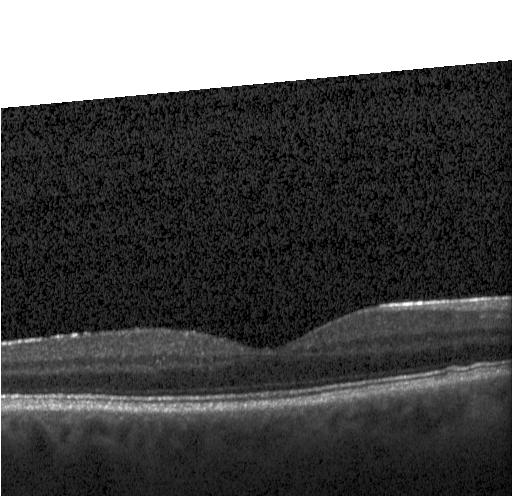

OCT line scan
The scan shows sub-RPE drusenoid deposits.